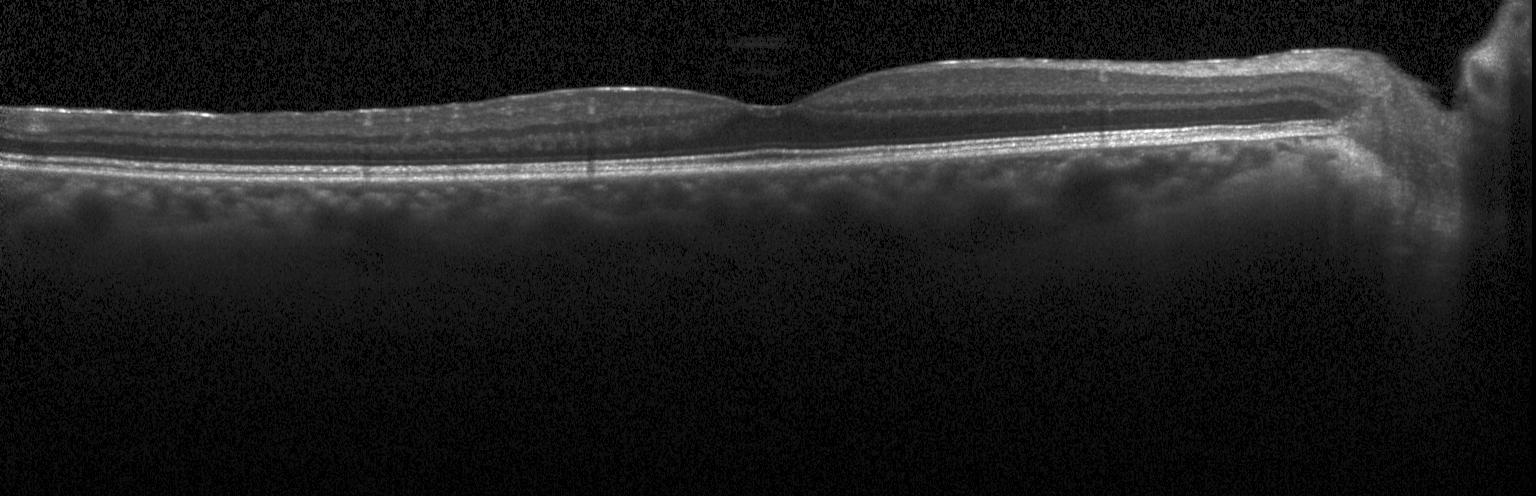 OCT B-scan showing no choroidal neovascularization, diabetic macular edema, or drusen.